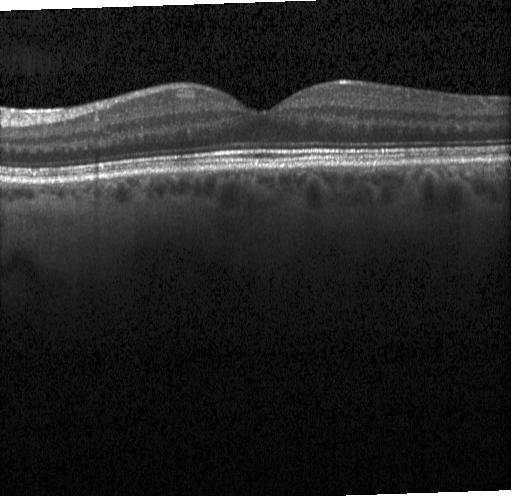
Optical coherence tomography B-scan. Impression: no CNV, no DME, and no drusen.